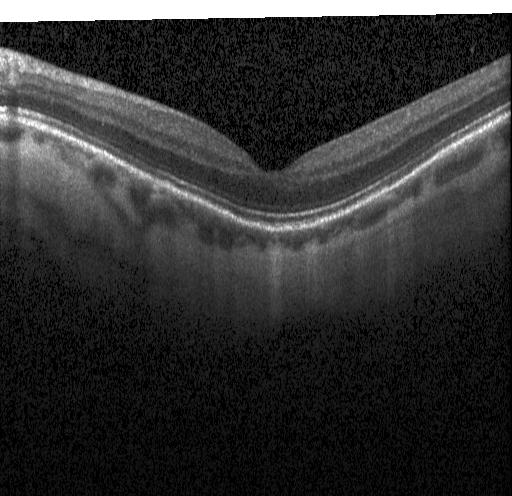 Optical coherence tomography scan. Through the macula. Heidelberg Spectralis. SD-OCT
Impression: no choroidal neovascularization, diabetic macular edema, or drusen.